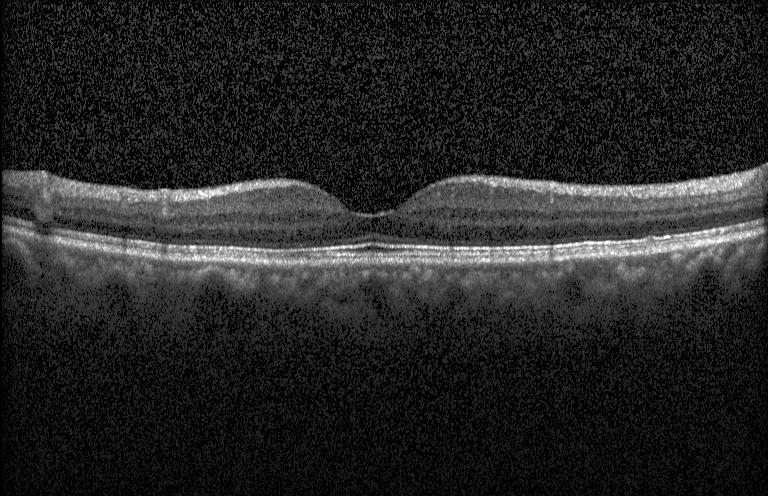
Optical coherence tomography scan. Diagnosis: neither CNV, DME, nor drusen.